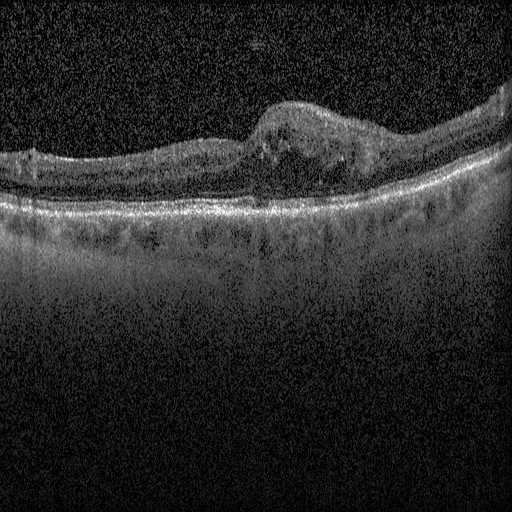 OCT B-scan; SD-OCT
Diabetic macular edema (DME).